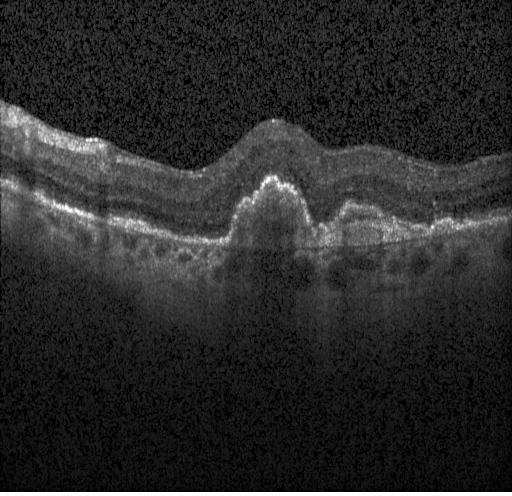
Retinal OCT B-scan — Impression: choroidal neovascularization (CNV).